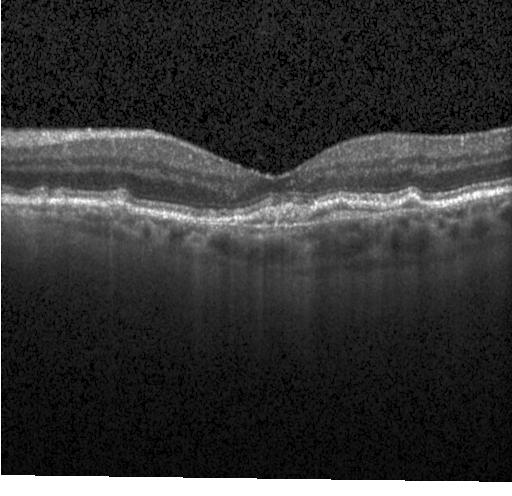
Heidelberg Spectralis. SD-OCT. Optical coherence tomography scan
Choroidal neovascularization.